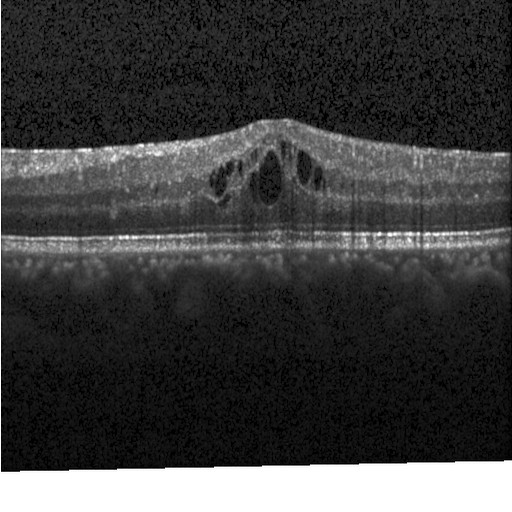 OCT B-scan showing diabetic macular edema.